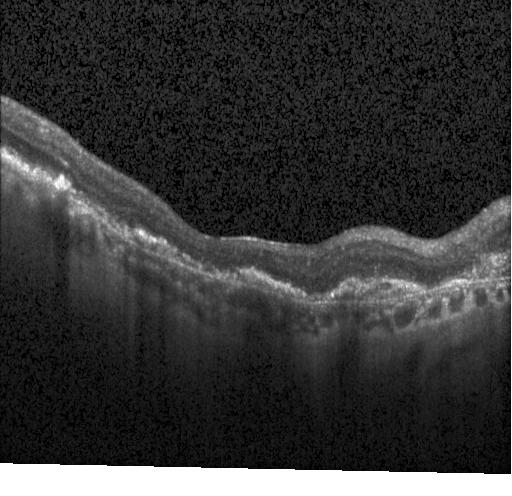
Retinal OCT cross-section showing choroidal neovascularization.